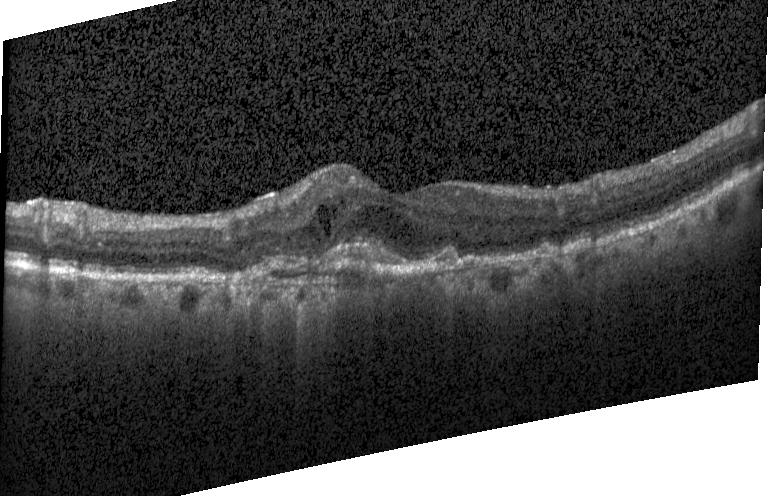
Optical coherence tomography scan
Finding: a choroidal neovascular membrane.